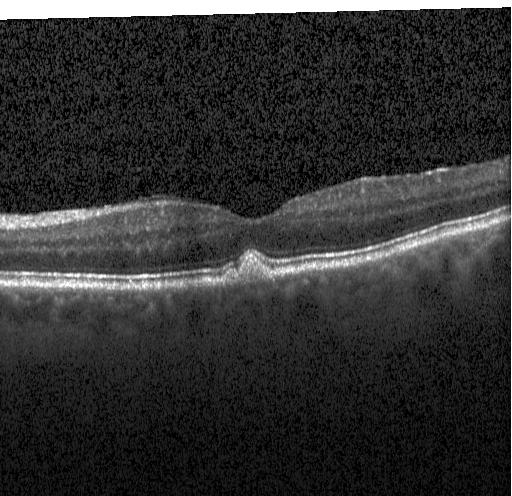

Retinal OCT cross-section showing multiple drusen.